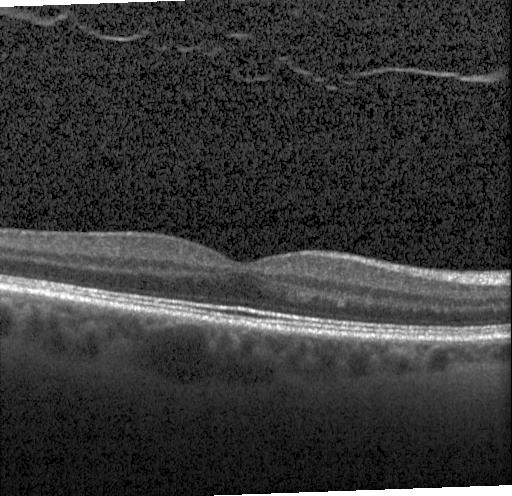 Retinal OCT cross-section; centered on the fovea
Macular OCT: no evidence of CNV, DME, or drusen.